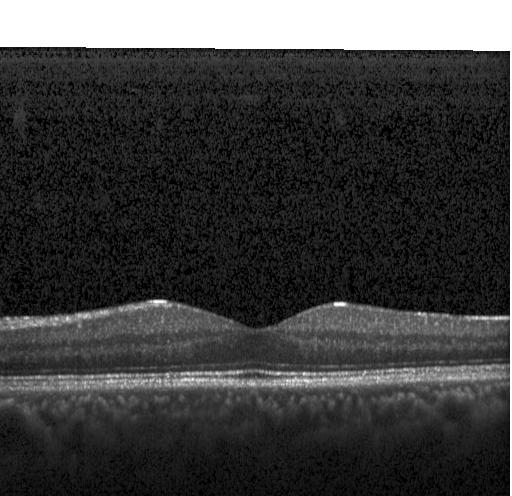 OCT B-scan — Impression: neither choroidal neovascularization, diabetic macular edema, nor drusen.